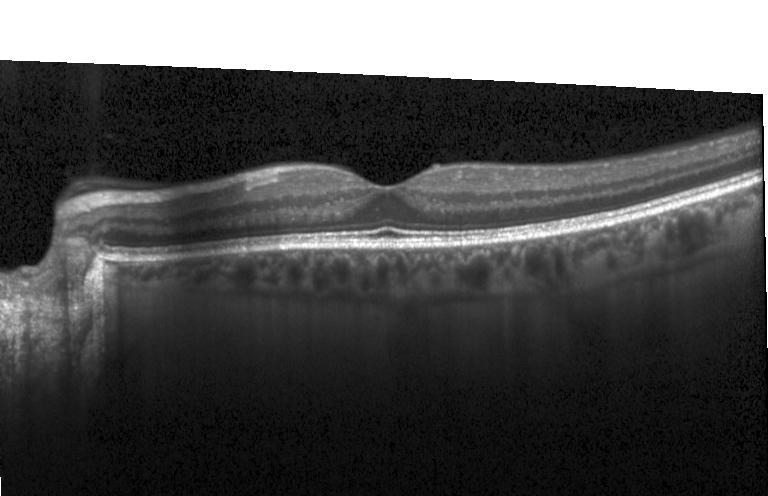

Diagnosis: no evidence of choroidal neovascularization, diabetic macular edema, or drusen.